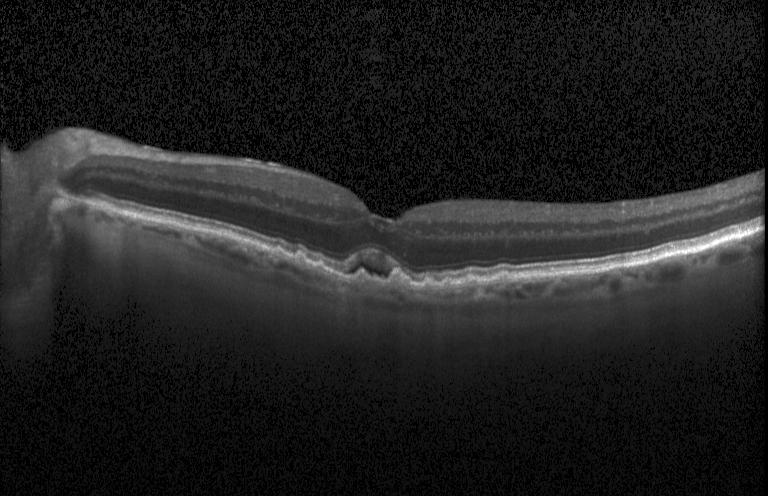

Optical coherence tomography scan; Heidelberg Spectralis.
Impression: a choroidal neovascular membrane.